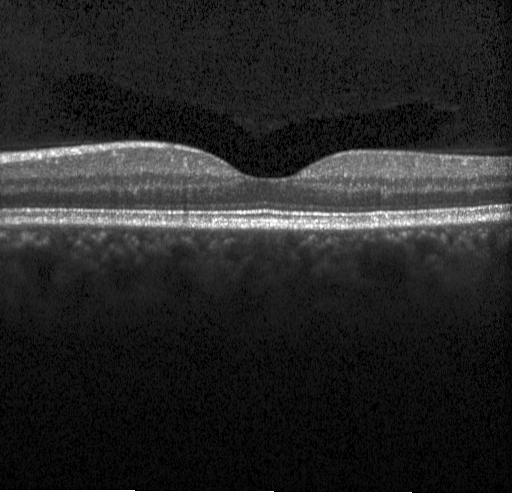
Retinal OCT B-scan. Instrument: Heidelberg Spectralis. Centered on the fovea. SD-OCT — Neither choroidal neovascularization, diabetic macular edema, nor drusen.